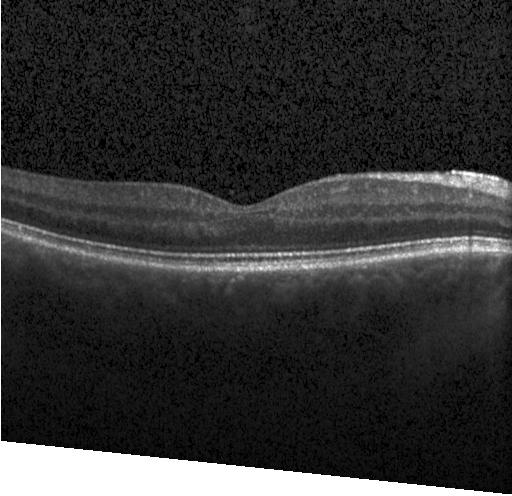 Acquired on a Heidelberg Spectralis. OCT line scan
This B-scan demonstrates no evidence of choroidal neovascularization, diabetic macular edema, or drusen.